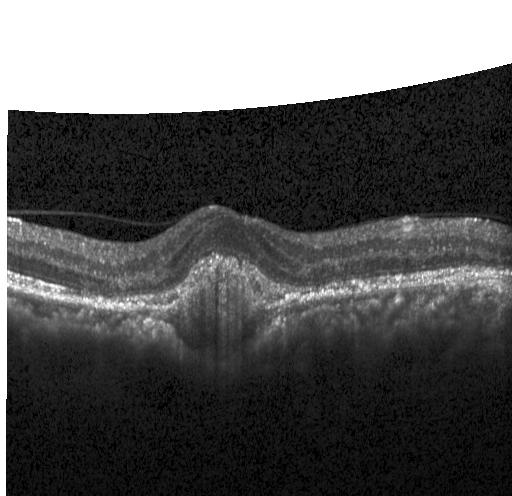
Spectral-domain OCT; retinal OCT B-scan; Heidelberg Spectralis OCT system; through the macula — Impression: a choroidal neovascular membrane.